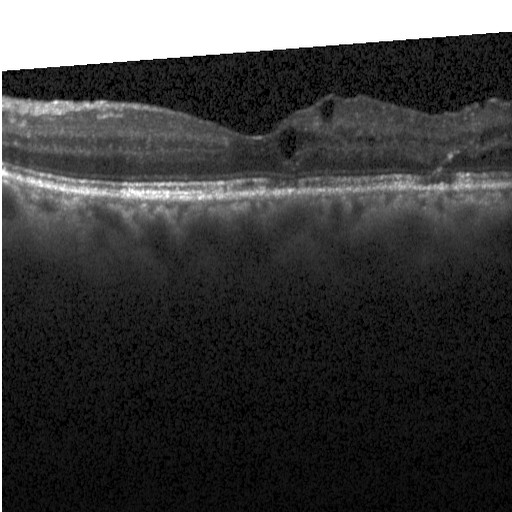 OCT scan showing diabetic macular edema.